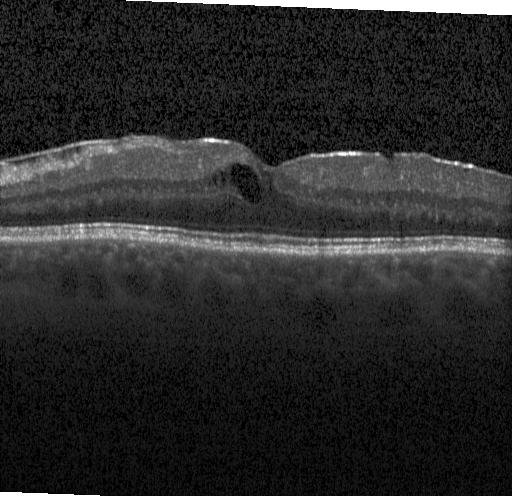
OCT finding: diabetic macular edema.